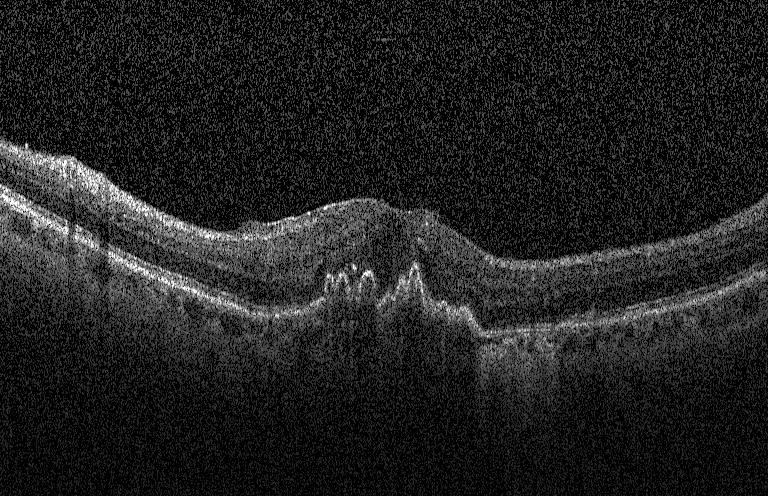
OCT line scan. Spectral-domain OCT. Horizontal scan through the fovea
OCT finding: a choroidal neovascular membrane.